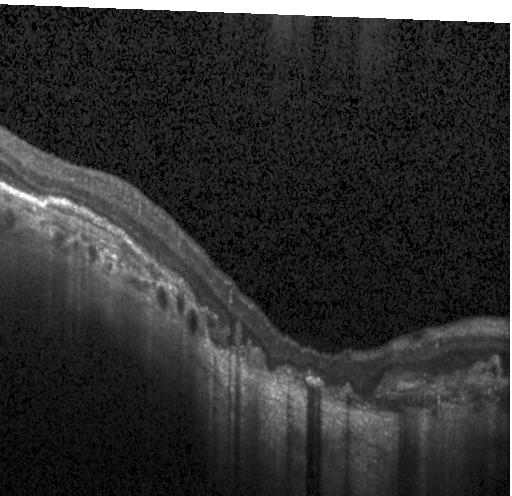 Spectral-domain OCT B-scan: a choroidal neovascular membrane.